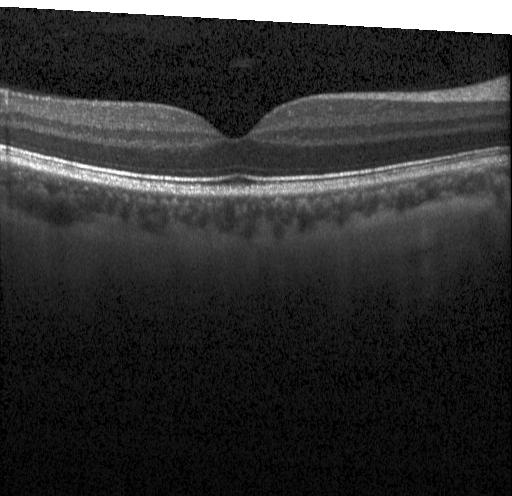 Finding: no choroidal neovascularization, no diabetic macular edema, and no drusen.